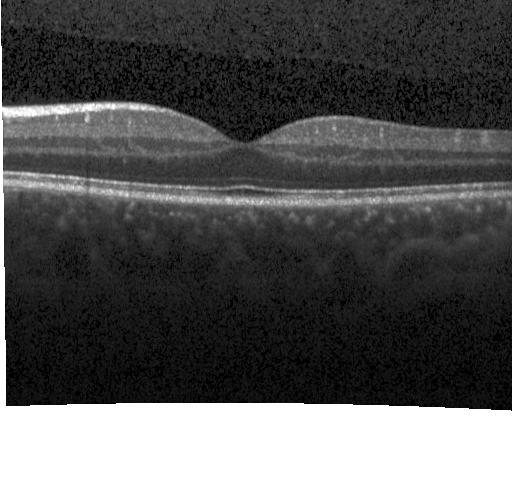

Spectral-domain OCT B-scan: no CNV, no DME, and no drusen.